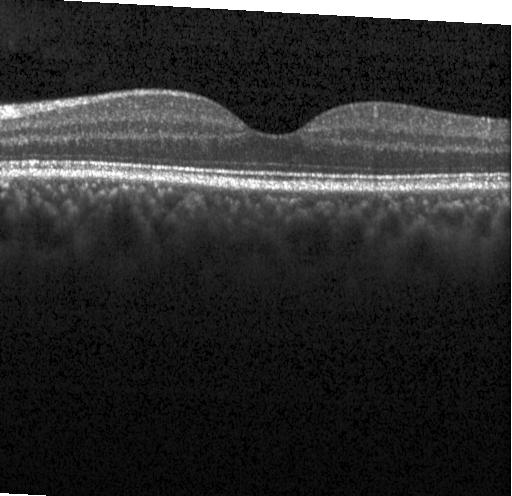

Optical coherence tomography scan.
OCT finding: neither choroidal neovascularization, diabetic macular edema, nor drusen.